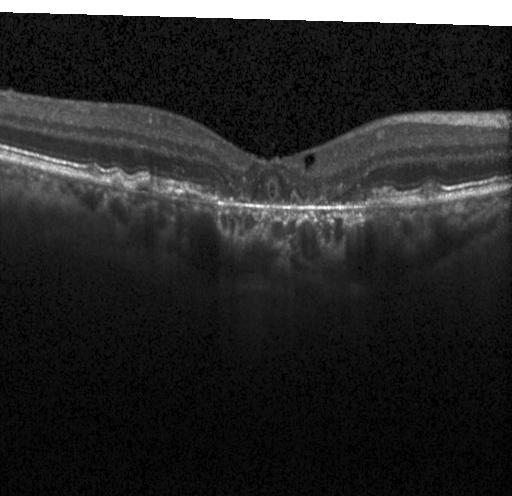
Optical coherence tomography scan. Finding: CNV.